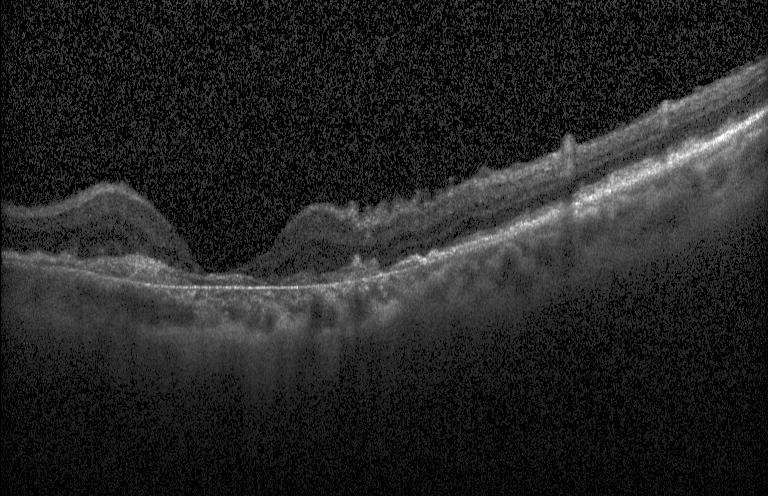 Assessment: a choroidal neovascular membrane.